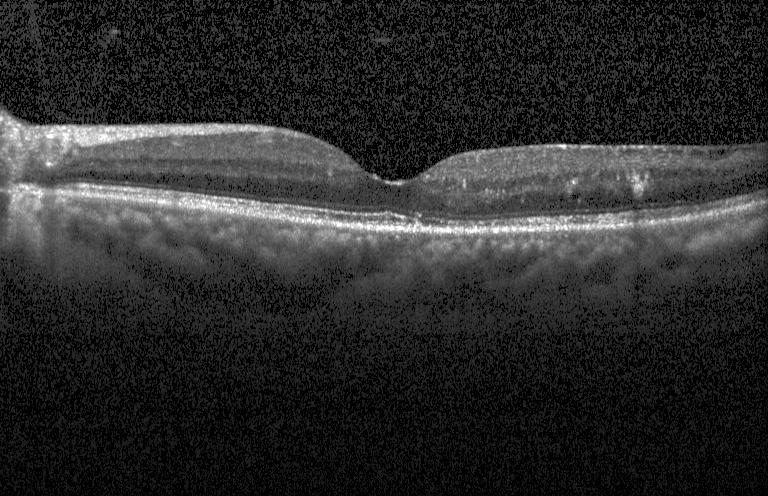 Heidelberg Spectralis OCT system · retinal OCT cross-section · spectral-domain OCT.
This B-scan demonstrates diabetic macular edema.